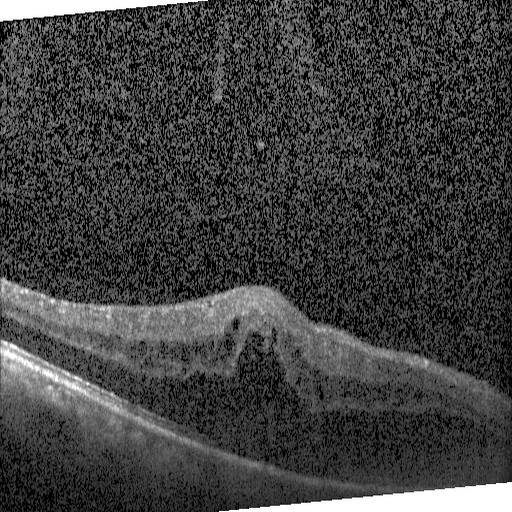
OCT B-scan. Finding: diabetic macular edema.